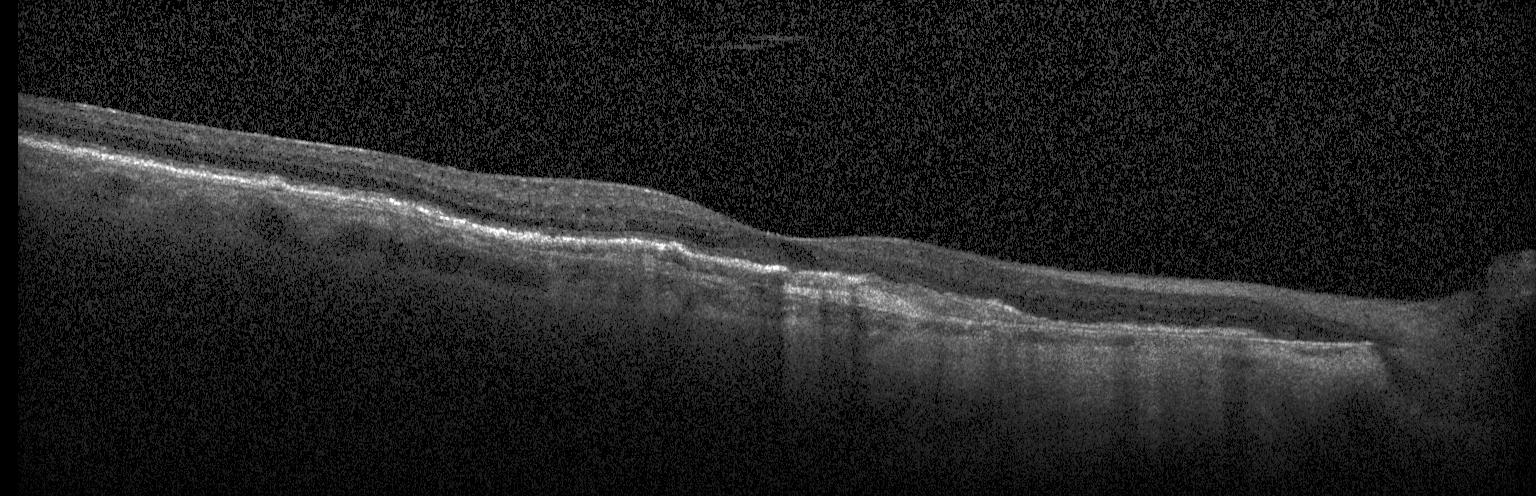 OCT line scan. Centered on the fovea
OCT finding: a choroidal neovascular membrane.